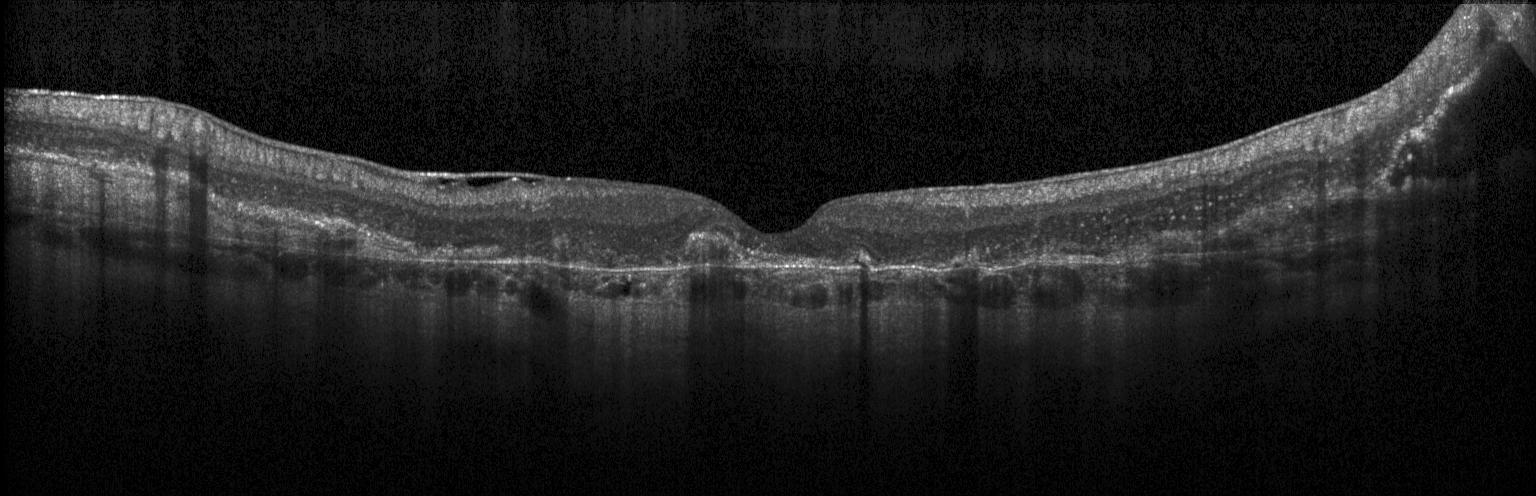
SD-OCT; OCT line scan; acquired on a Heidelberg Spectralis. Diagnosis: a choroidal neovascular membrane.